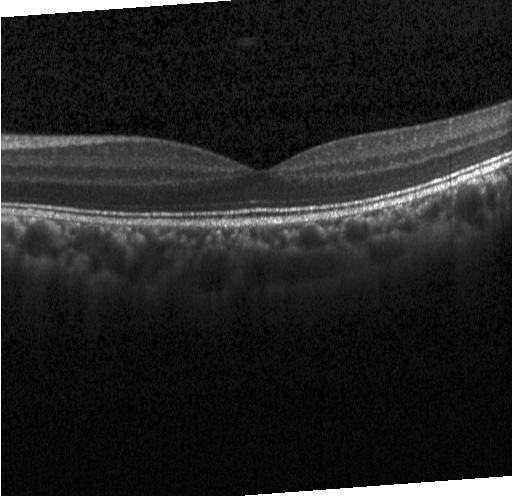

Optical coherence tomography B-scan
Macular OCT: no choroidal neovascularization, no diabetic macular edema, and no drusen.